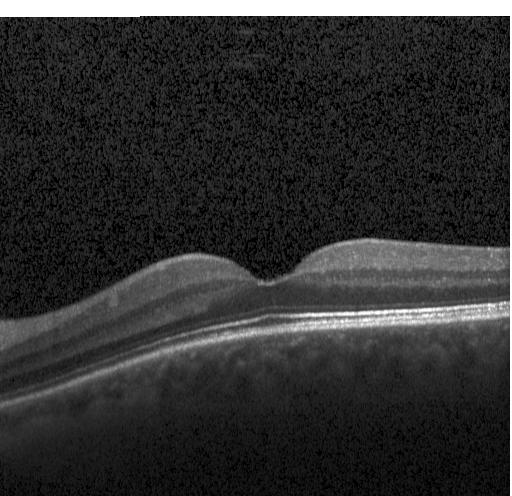 OCT finding: no evidence of choroidal neovascularization, diabetic macular edema, or drusen.